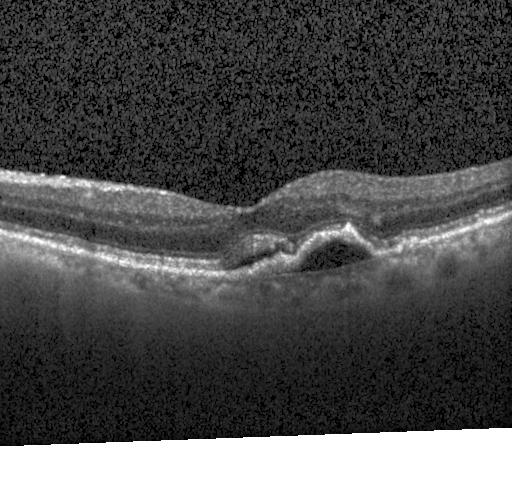

Heidelberg Spectralis · retinal OCT cross-section · macular scan · spectral-domain OCT. Finding: choroidal neovascularization.